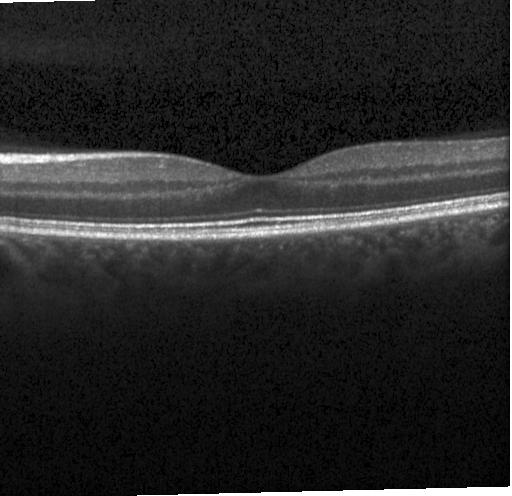 Instrument: Heidelberg Spectralis. Fovea-centered. Spectral-domain OCT. Optical coherence tomography scan — Diagnosis: no CNV, no DME, and no drusen.